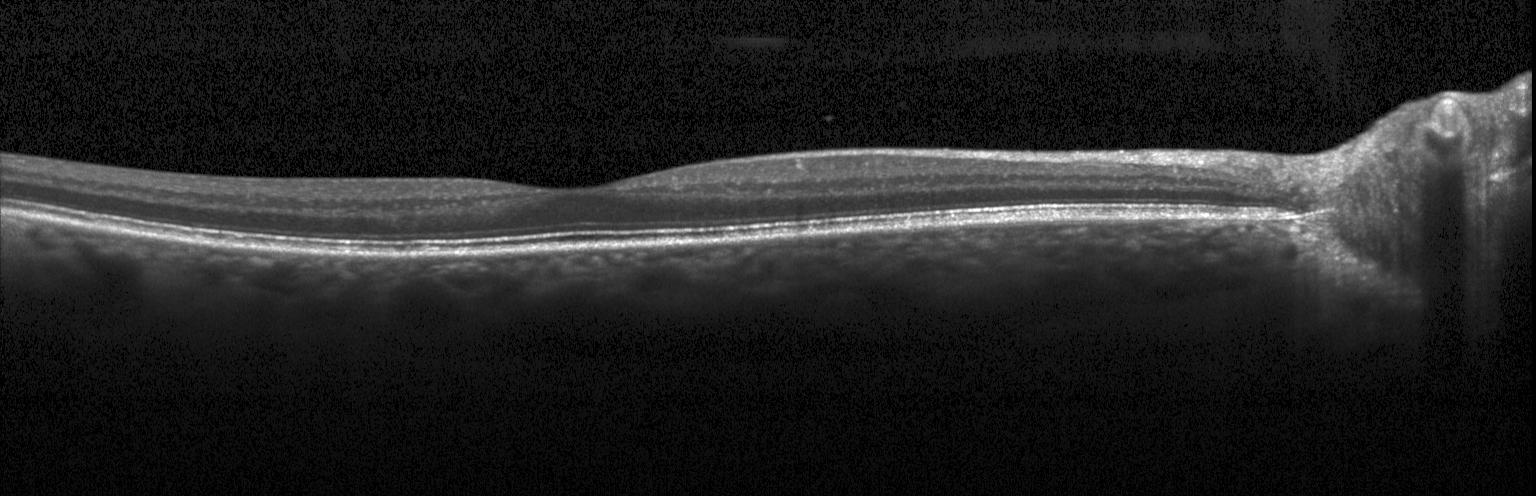

Optical coherence tomography scan, SD-OCT, through the macula
The scan shows no choroidal neovascularization, no diabetic macular edema, and no drusen.